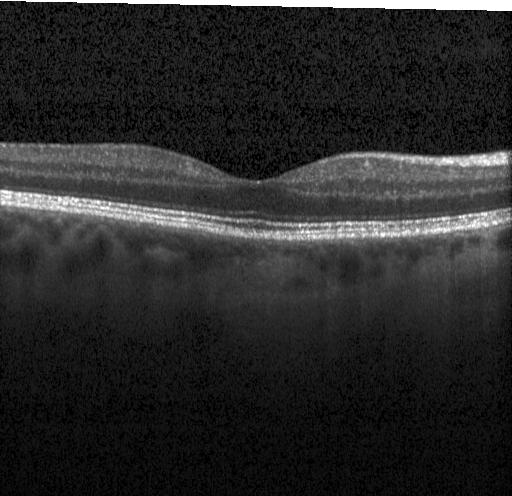 OCT B-scan showing neither choroidal neovascularization, diabetic macular edema, nor drusen.